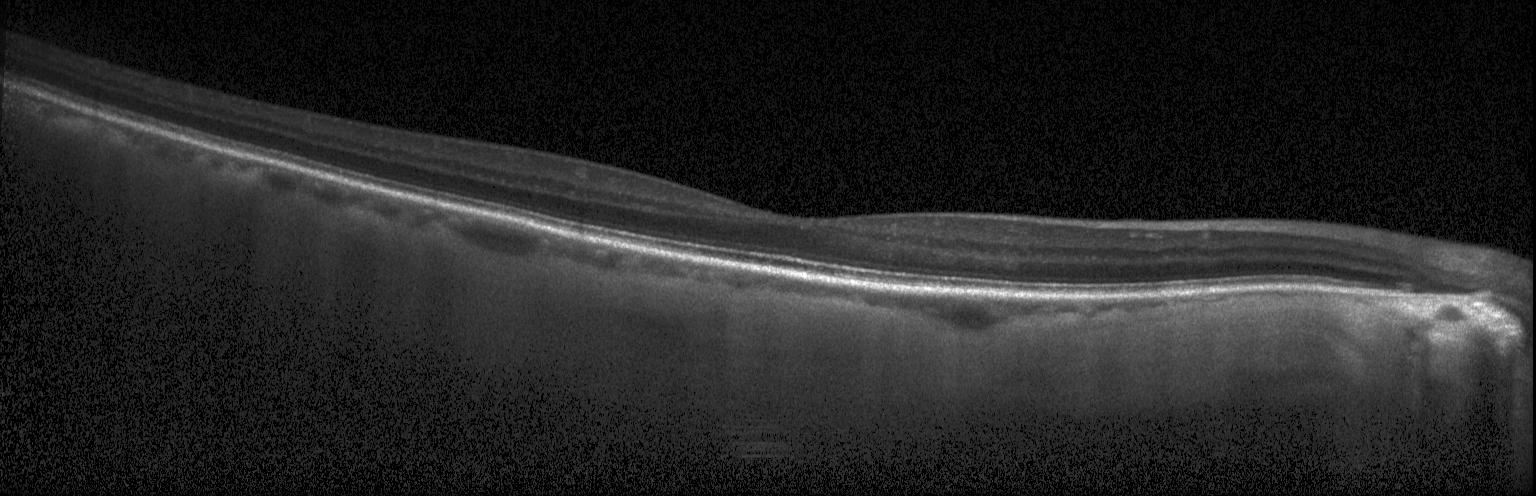

Macular OCT: no CNV, DME, or drusen.